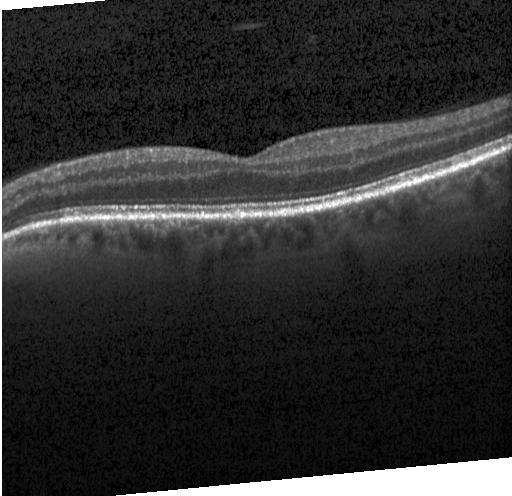 OCT B-scan showing no evidence of choroidal neovascularization, diabetic macular edema, or drusen.